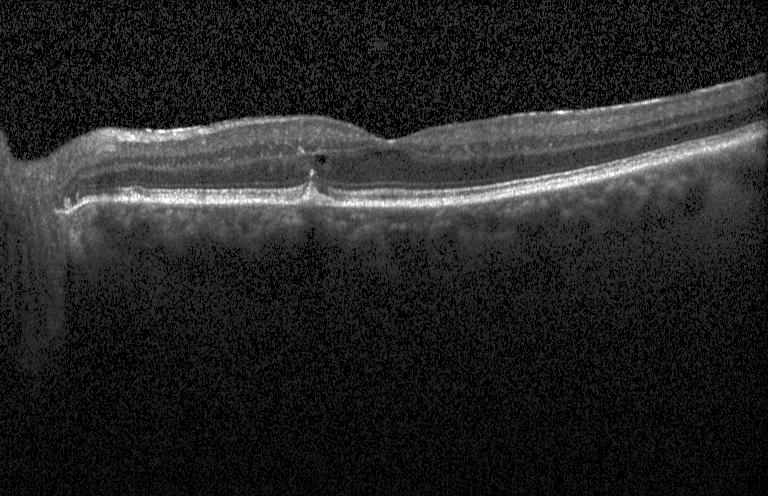

Instrument: Heidelberg Spectralis; optical coherence tomography scan. Impression: choroidal neovascularization.